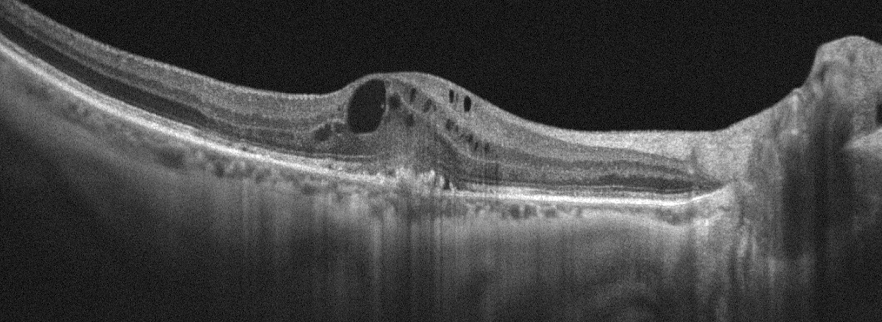
Optical coherence tomography B-scan · oculus dexter
Assessment: age-related macular degeneration.